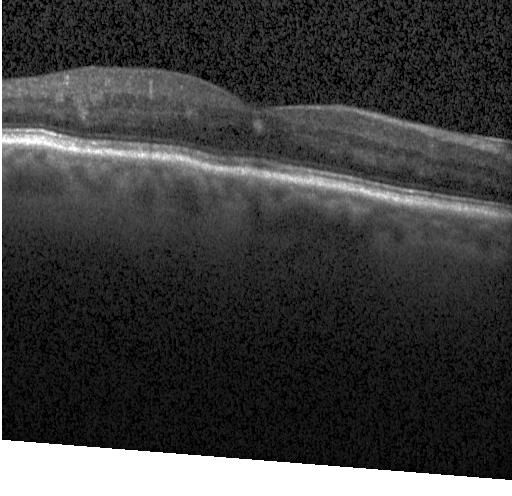 Diagnosis: no choroidal neovascularization, diabetic macular edema, or drusen.